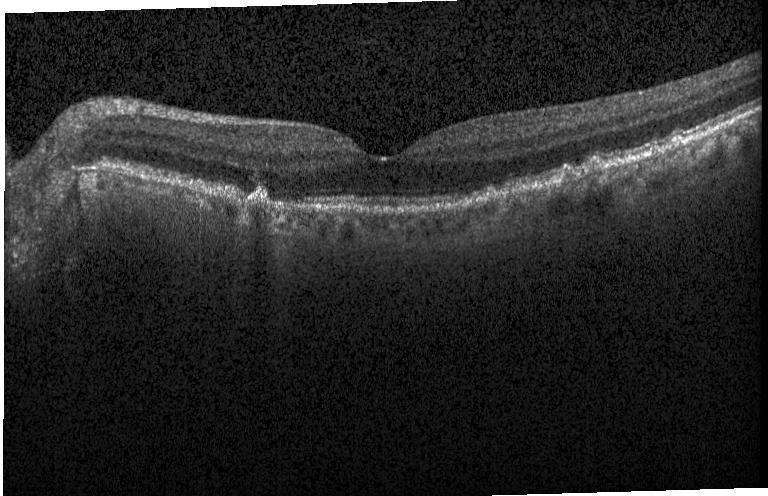

Heidelberg Spectralis. OCT B-scan
Macular OCT: drusen.